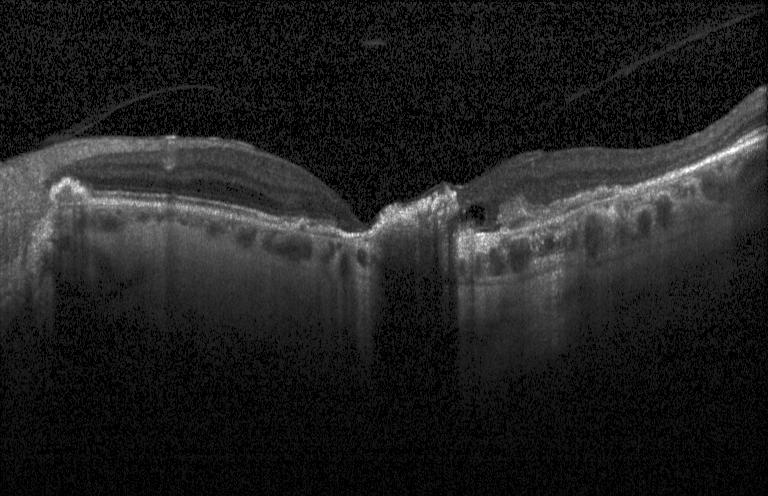
Spectral-domain optical coherence tomography · optical coherence tomography scan · instrument: Heidelberg Spectralis · fovea-centered. The scan shows choroidal neovascularization.